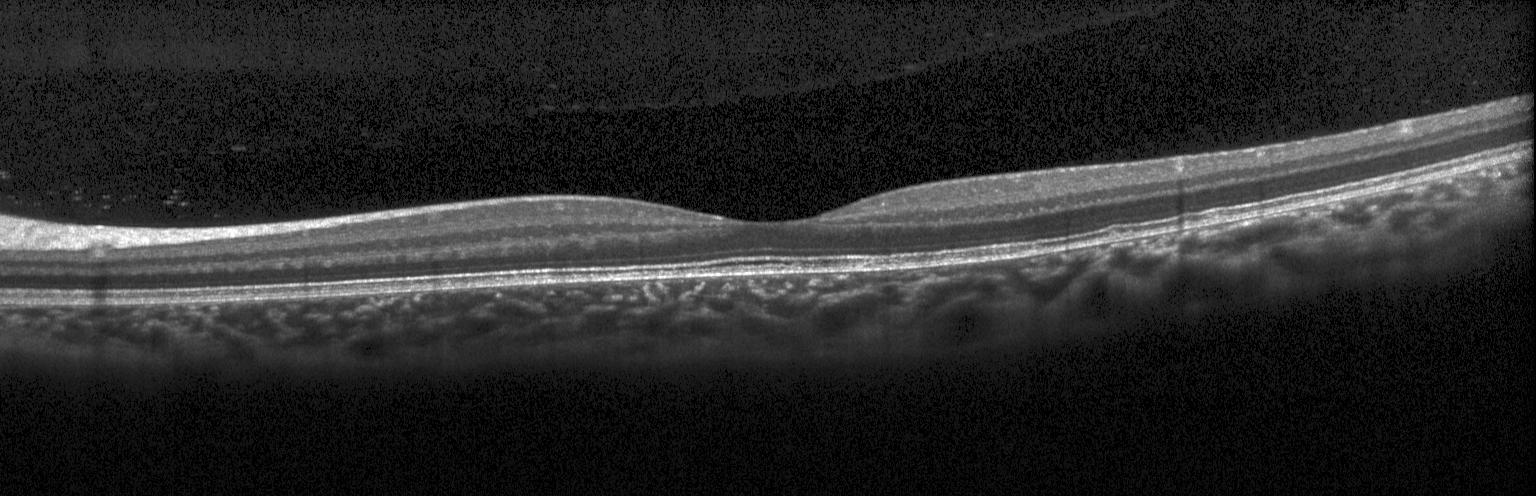 Retinal OCT cross-section
Assessment: neither CNV, DME, nor drusen.